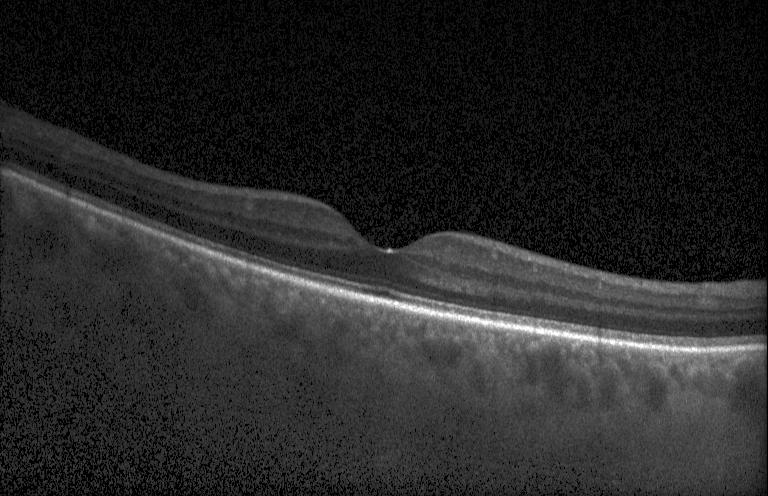 OCT B-scan
Diagnosis: neither CNV, DME, nor drusen.